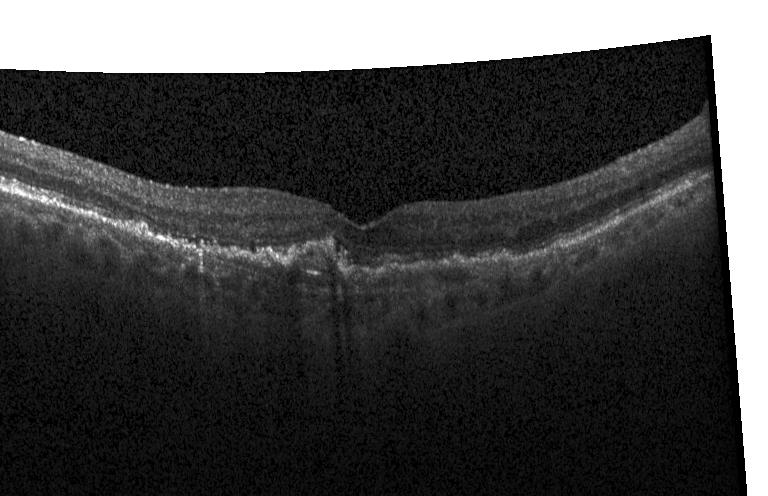
Heidelberg Spectralis; macular scan; spectral-domain OCT; retinal OCT cross-section
OCT finding: choroidal neovascularization.